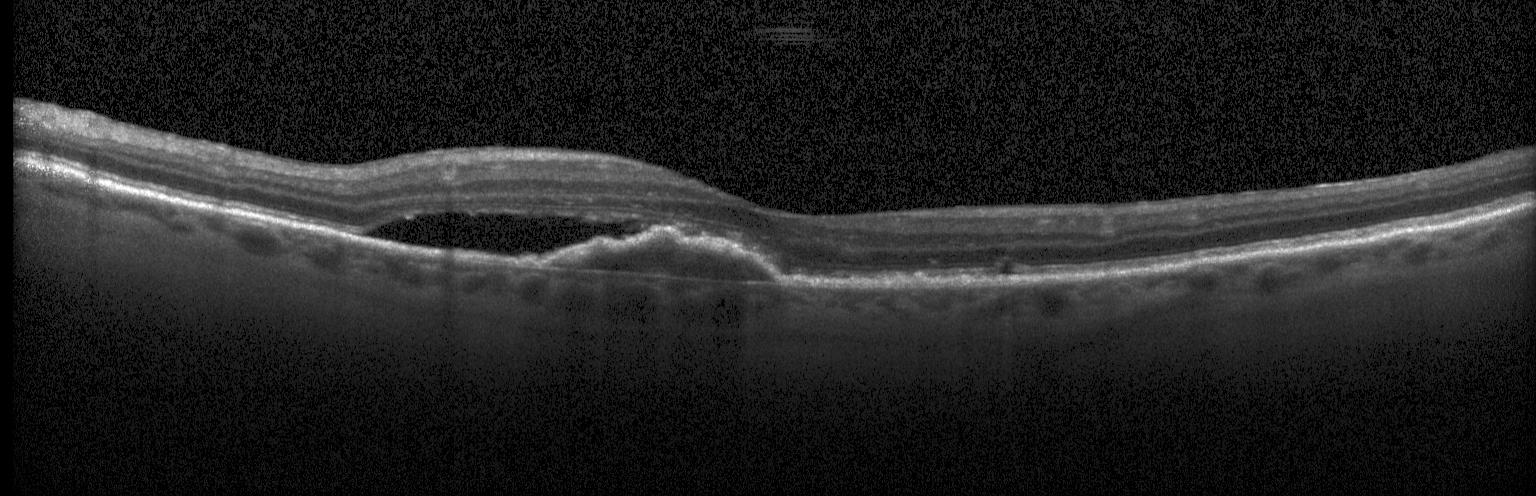
Optical coherence tomography scan · horizontal scan through the fovea.
OCT finding: a choroidal neovascular membrane.